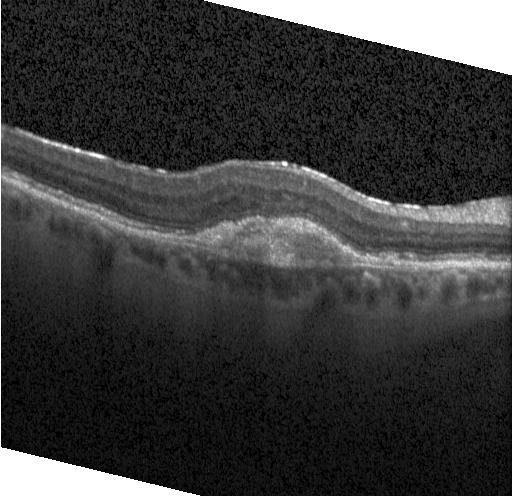 Retinal OCT cross-section showing choroidal neovascularization (CNV).